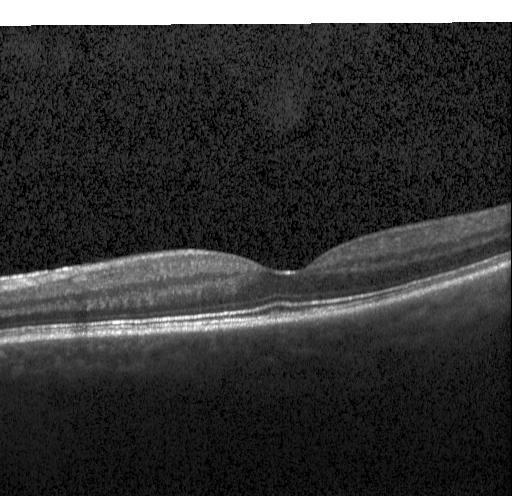 SD-OCT · retinal OCT cross-section · fovea-centered · Heidelberg Spectralis — Diagnosis: neither CNV, DME, nor drusen.